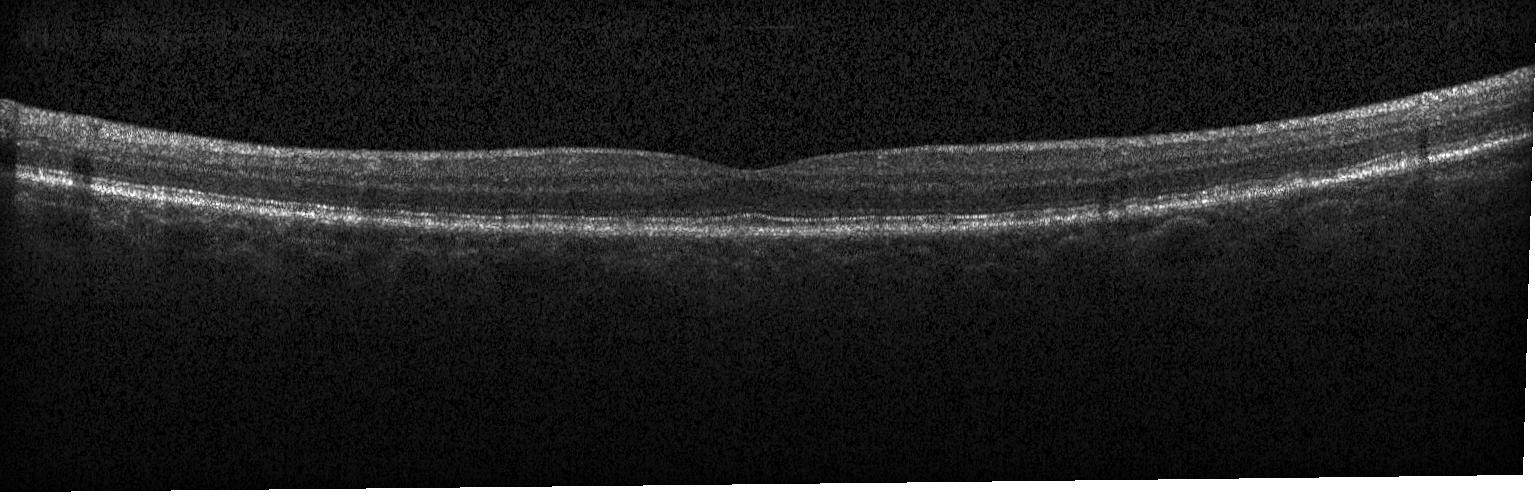

Assessment: sub-RPE drusenoid deposits.